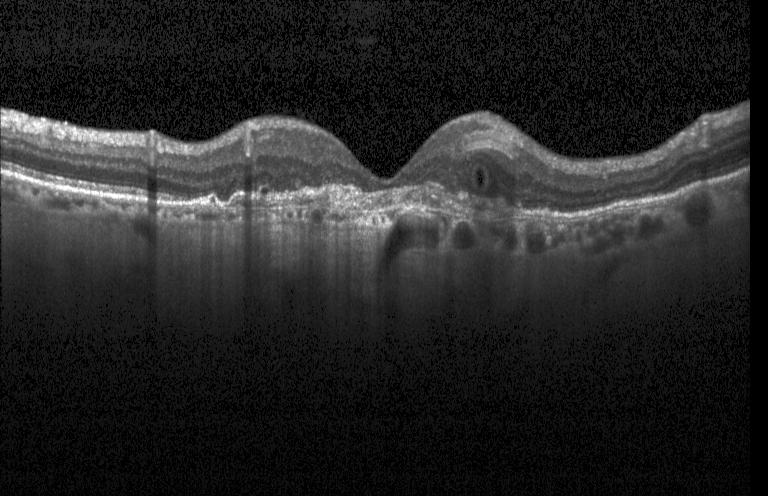

Finding: a choroidal neovascular membrane.